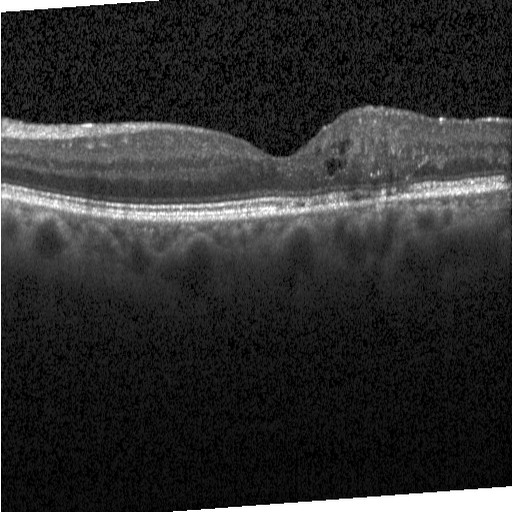
SD-OCT. Horizontal scan through the fovea. OCT line scan — Diagnosis: diabetic macular edema (DME).